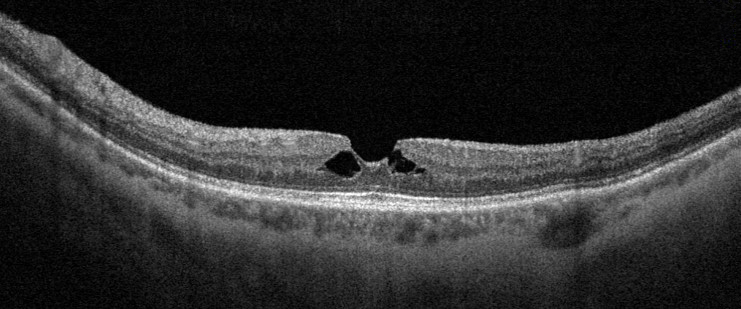
Instrument: Optovue Avanti RTVue XR · retinal OCT cross-section · macular scan
Diagnosis: vitreomacular interface disease.